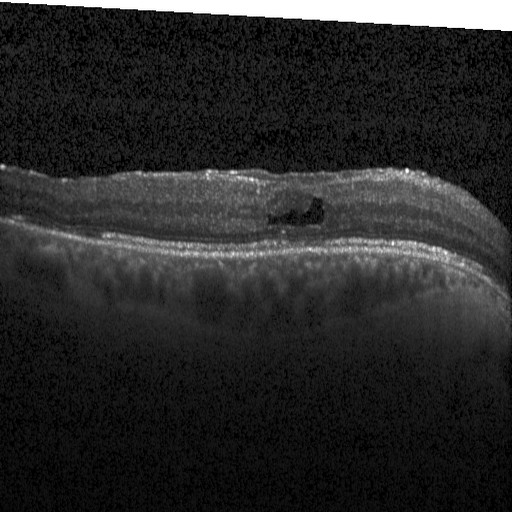

Optical coherence tomography B-scan. Instrument: Heidelberg Spectralis. Horizontal scan through the fovea. Spectral-domain OCT. Impression: diabetic macular edema.